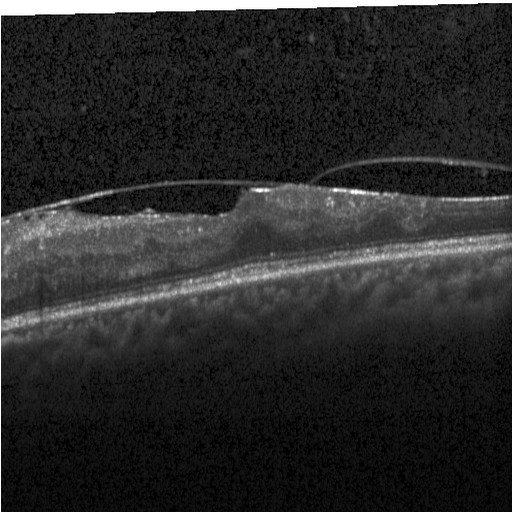
Optical coherence tomography B-scan, centered on the fovea, instrument: Heidelberg Spectralis. OCT finding: diabetic macular edema.